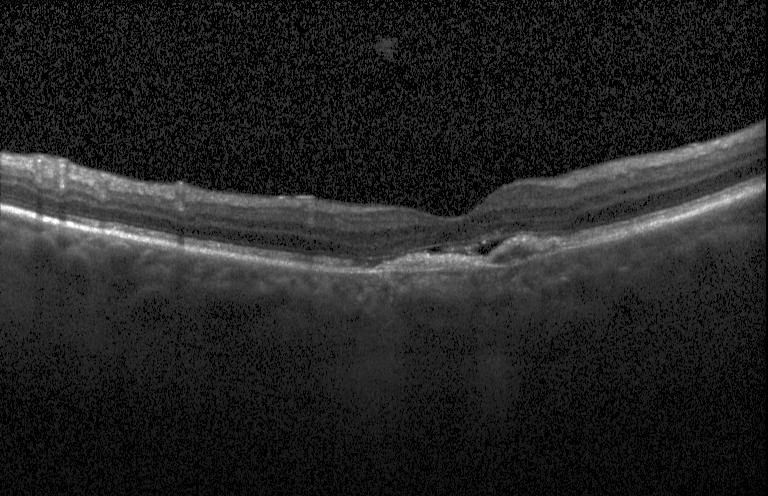

OCT finding: CNV.